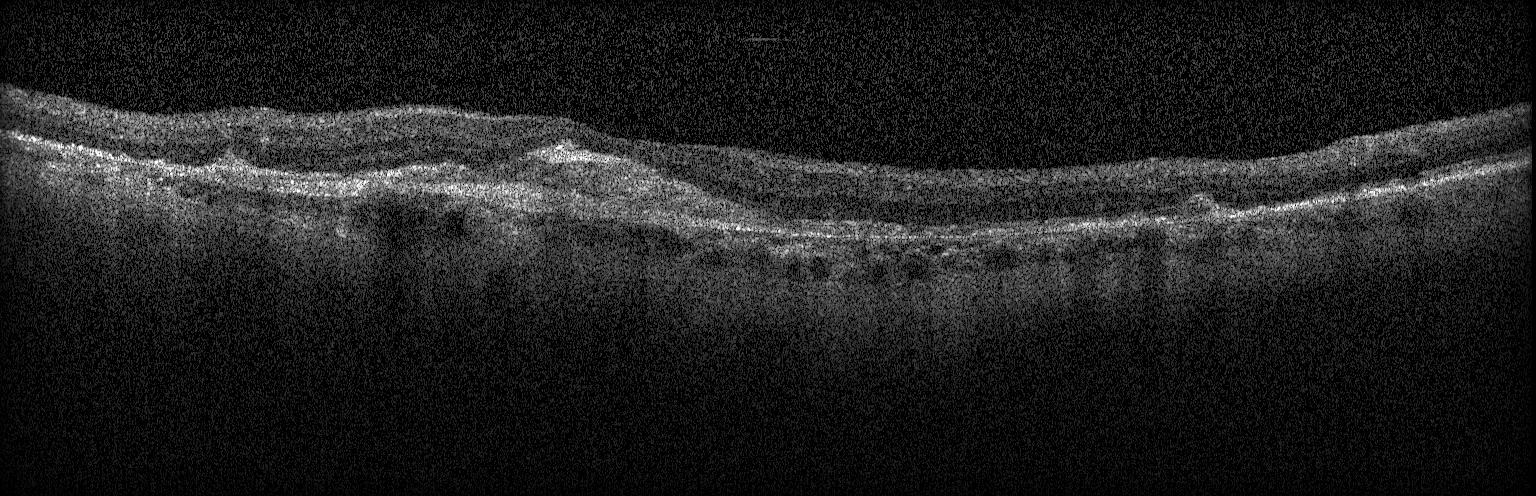
Optical coherence tomography B-scan; spectral-domain optical coherence tomography. Finding: a choroidal neovascular membrane.